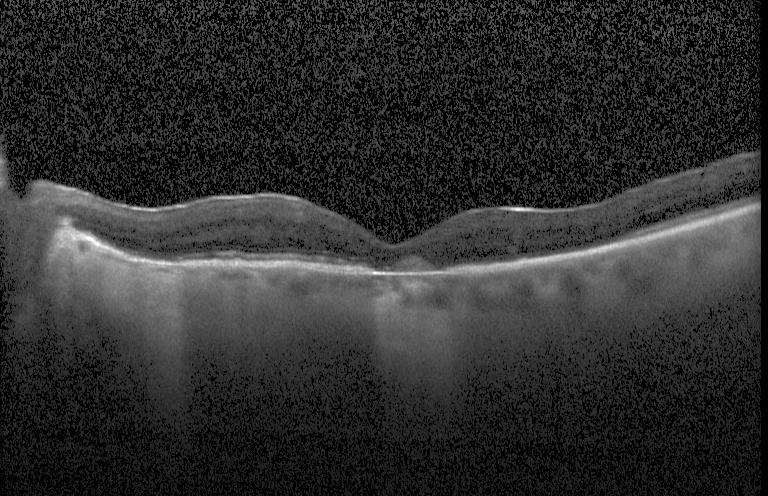

The scan shows CNV.